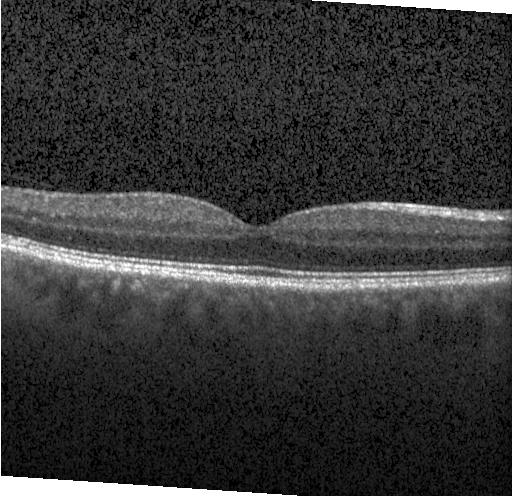

Diagnosis: no CNV, DME, or drusen.